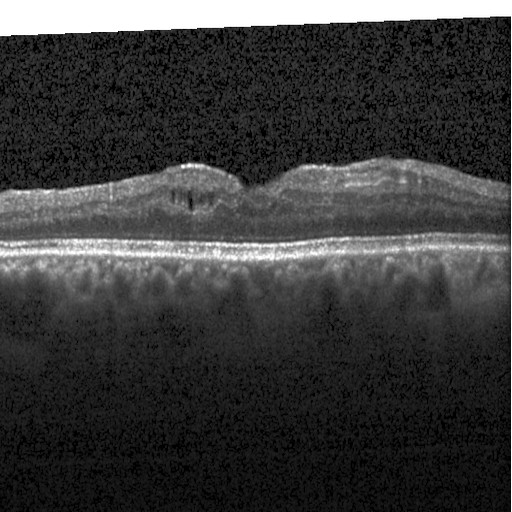
Macular OCT demonstrating DME.